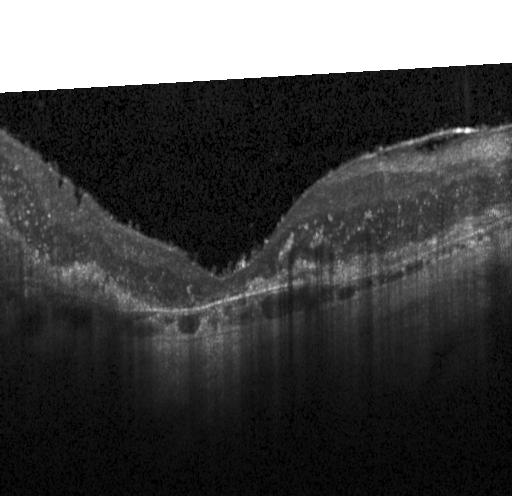
OCT B-scan, instrument: Heidelberg Spectralis, spectral-domain optical coherence tomography — OCT finding: a choroidal neovascular membrane.